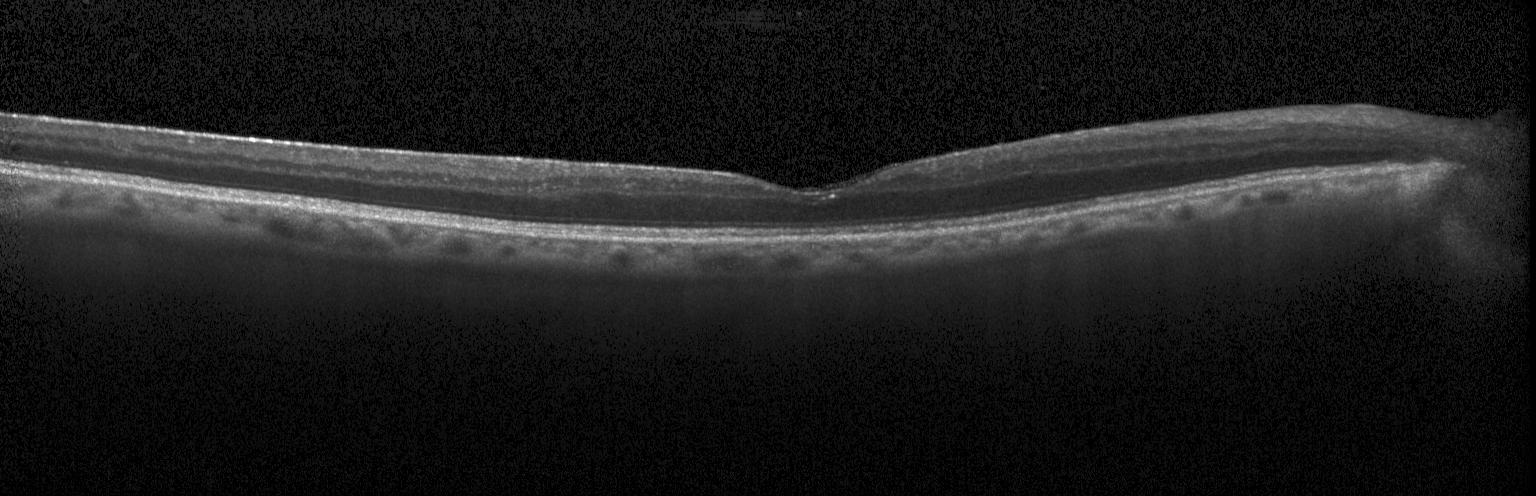

OCT B-scan showing no choroidal neovascularization, diabetic macular edema, or drusen.